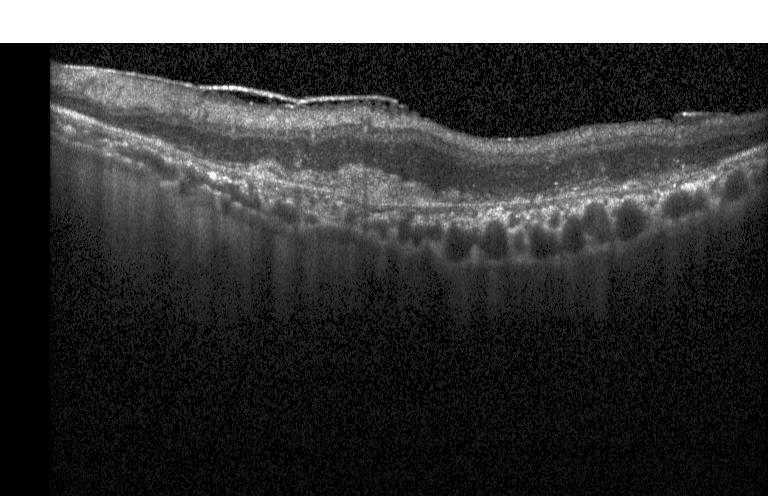 Retinal OCT cross-section; Heidelberg Spectralis.
Macular OCT: a choroidal neovascular membrane.